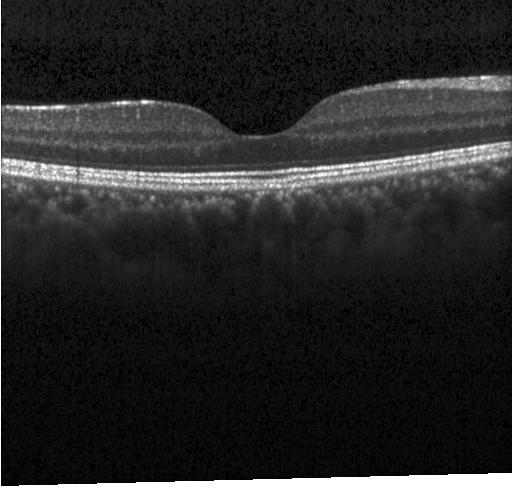

OCT B-scan
Impression: no evidence of choroidal neovascularization, diabetic macular edema, or drusen.